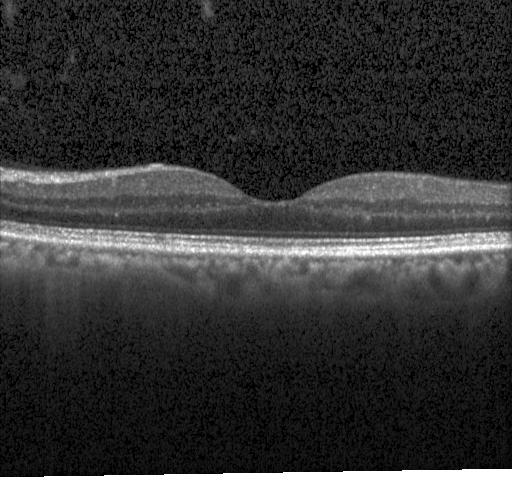

Diagnosis: no evidence of choroidal neovascularization, diabetic macular edema, or drusen.